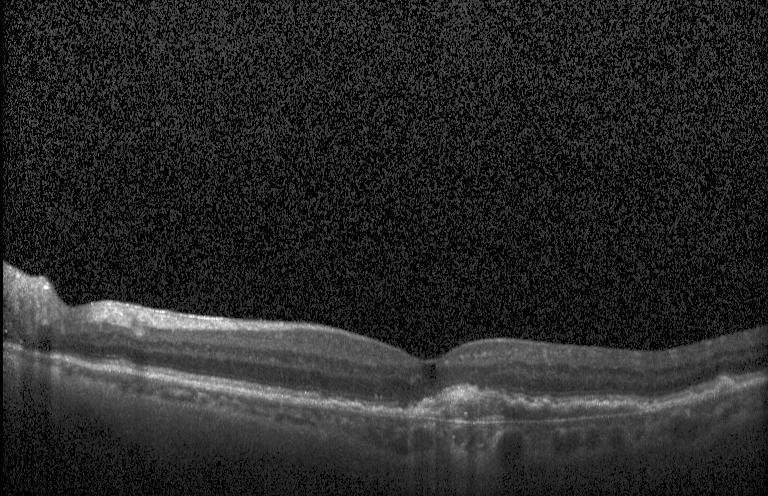

Optical coherence tomography scan; Heidelberg Spectralis; macular scan — Impression: a choroidal neovascular membrane.